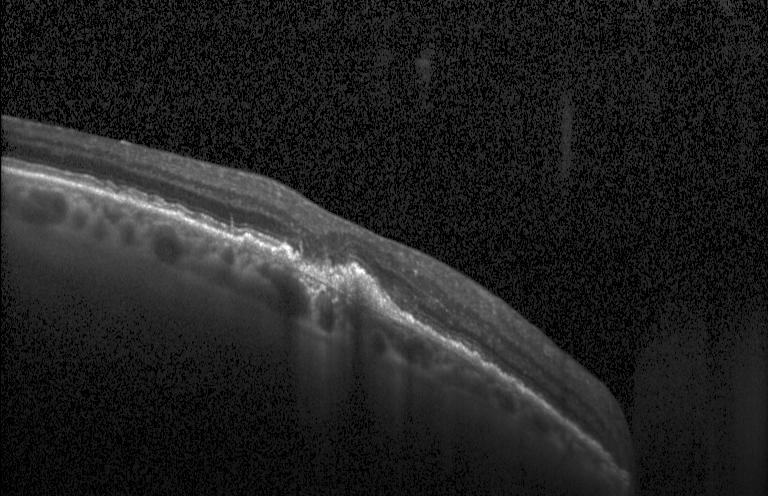 Diagnosis: CNV.